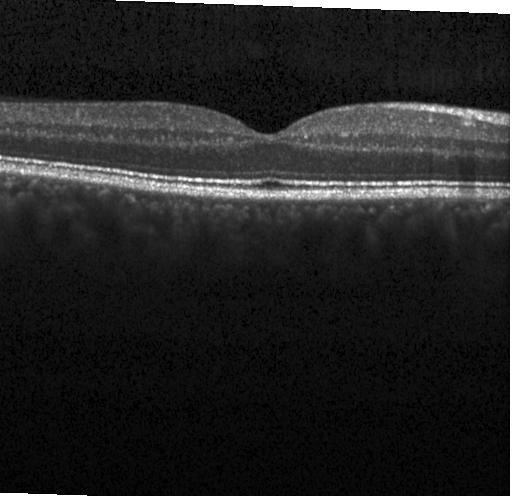
Heidelberg Spectralis, macular scan, spectral-domain OCT, retinal OCT B-scan.
OCT finding: no choroidal neovascularization, diabetic macular edema, or drusen.